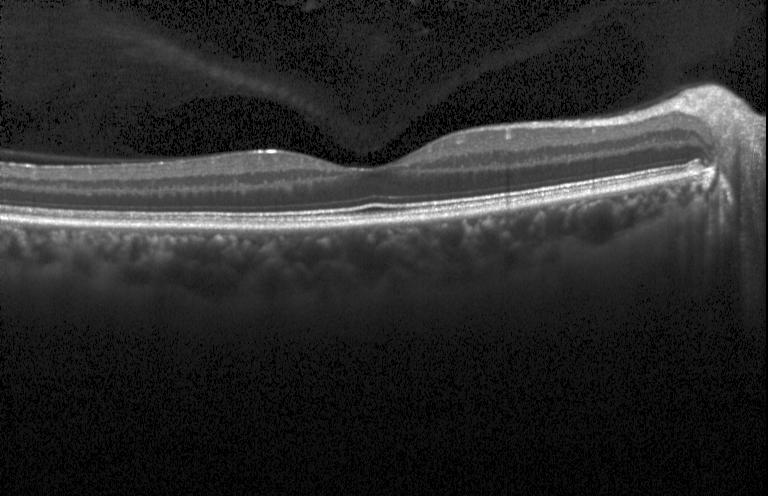

Fovea-centered · SD-OCT · OCT line scan · Heidelberg Spectralis OCT system.
This B-scan demonstrates no choroidal neovascularization, diabetic macular edema, or drusen.